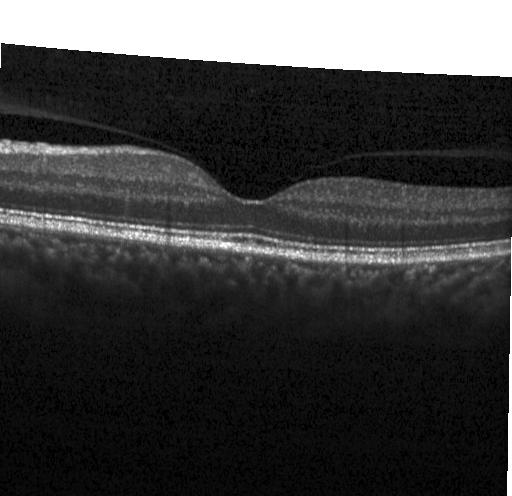

Spectral-domain OCT; through the macula; acquired on a Heidelberg Spectralis; OCT line scan — Diagnosis: no evidence of CNV, DME, or drusen.